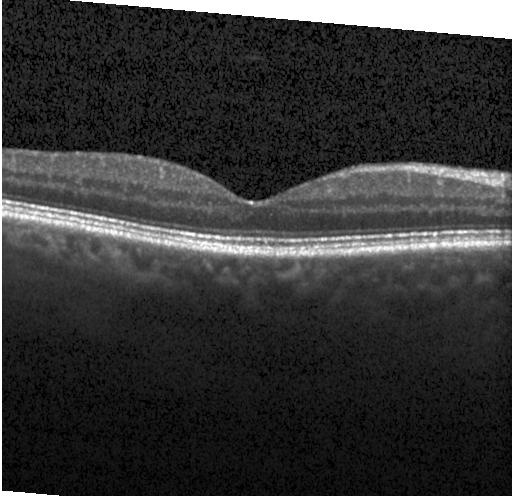

OCT B-scan; instrument: Heidelberg Spectralis. Impression: neither choroidal neovascularization, diabetic macular edema, nor drusen.